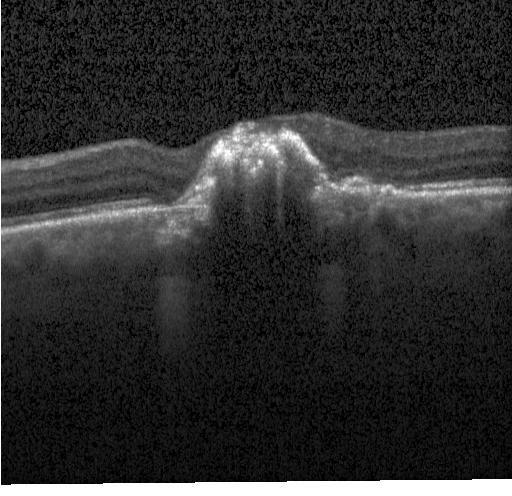 Impression: choroidal neovascularization.